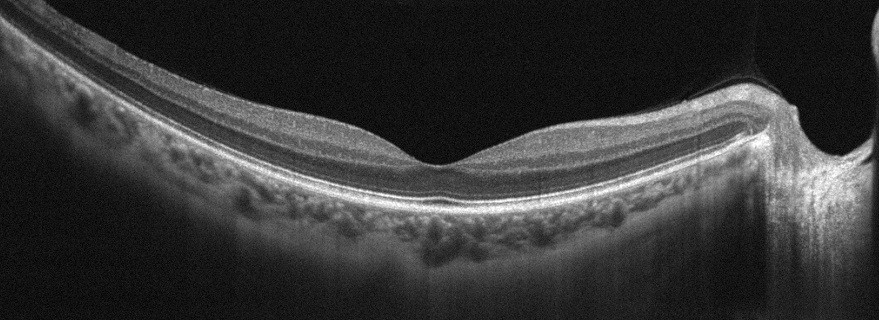

OCT scan showing no AMD, DME, ERM, RAO, RVO, or VID.